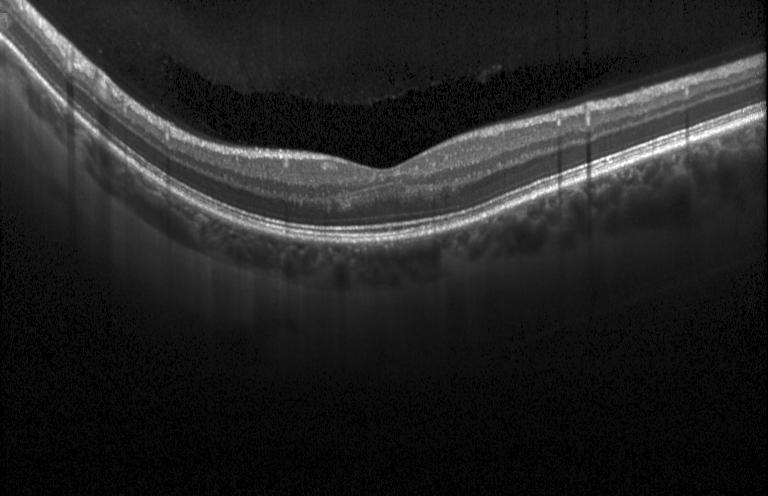

Macular OCT: no choroidal neovascularization, no diabetic macular edema, and no drusen.